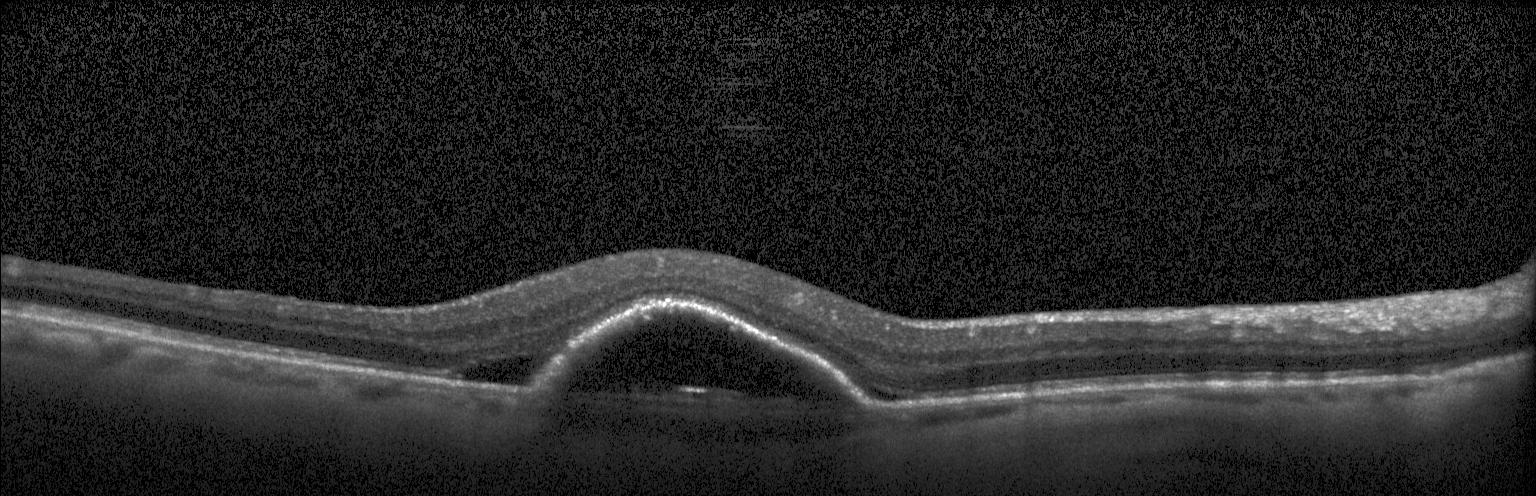 Finding: a choroidal neovascular membrane.